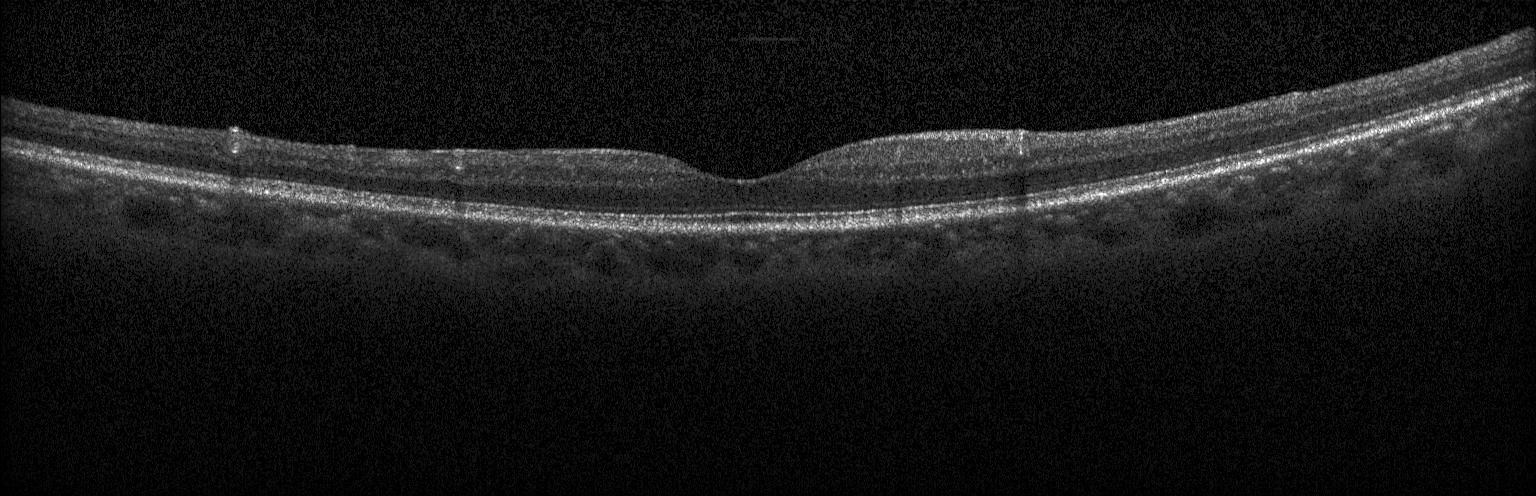

Retinal OCT cross-section. Through the macula. Macular OCT: no evidence of choroidal neovascularization, diabetic macular edema, or drusen.